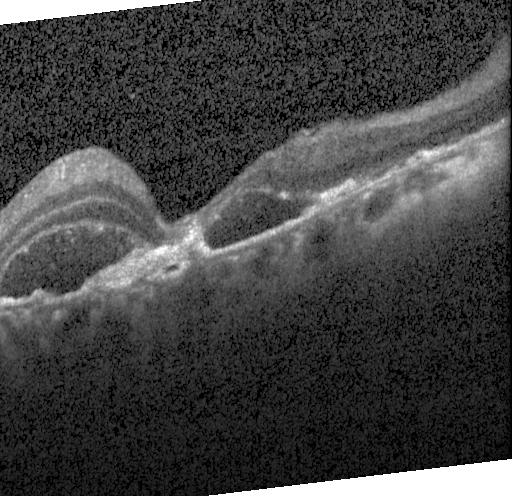

Macular OCT demonstrating choroidal neovascularization (CNV).